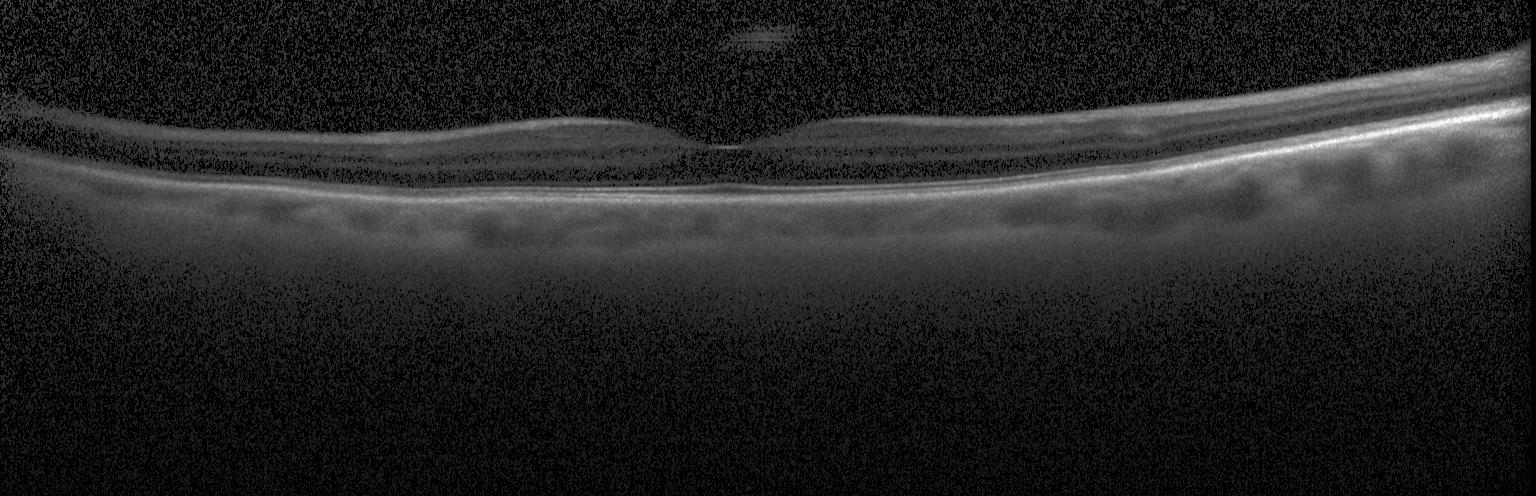
Optical coherence tomography B-scan. Macular OCT: no evidence of CNV, DME, or drusen.